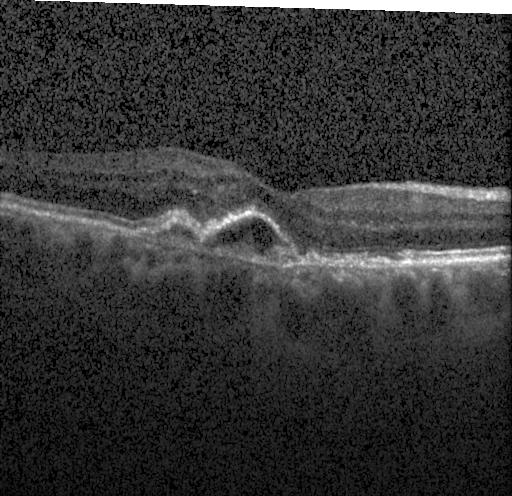

Centered on the fovea · optical coherence tomography B-scan
The scan shows CNV.